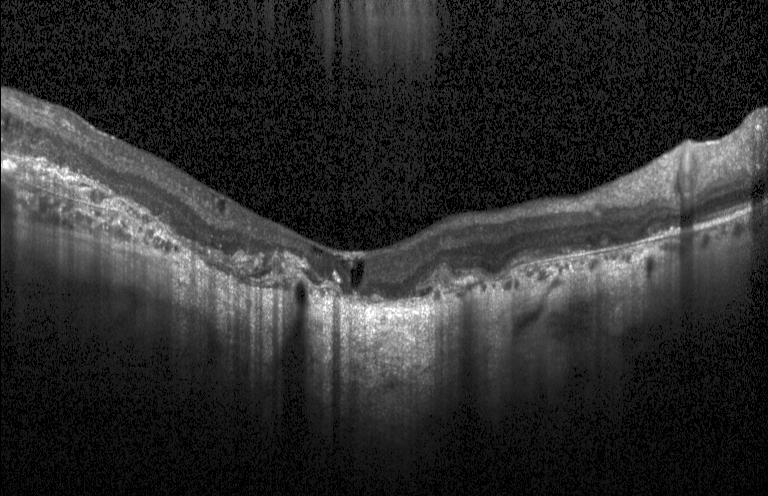 Instrument: Heidelberg Spectralis, OCT line scan, SD-OCT. Diagnosis: a choroidal neovascular membrane.